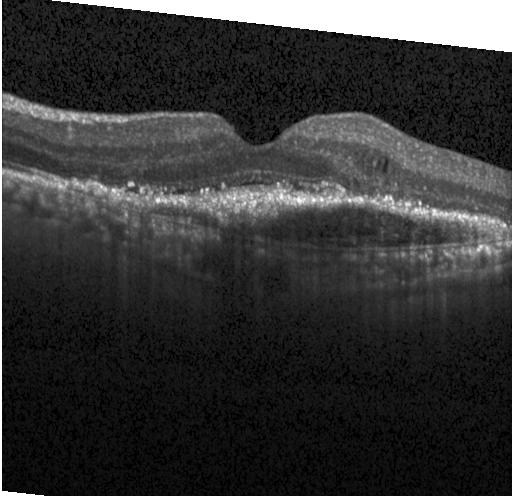
Acquired on a Heidelberg Spectralis, optical coherence tomography B-scan.
The scan shows choroidal neovascularization.